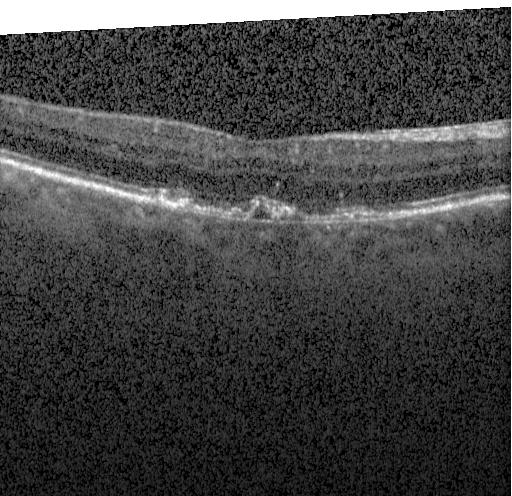 Retinal OCT cross-section showing a choroidal neovascular membrane.